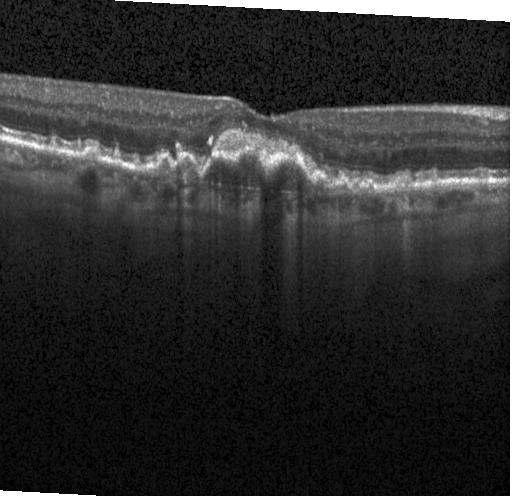

Retinal OCT B-scan; fovea-centered; SD-OCT — Finding: a choroidal neovascular membrane.